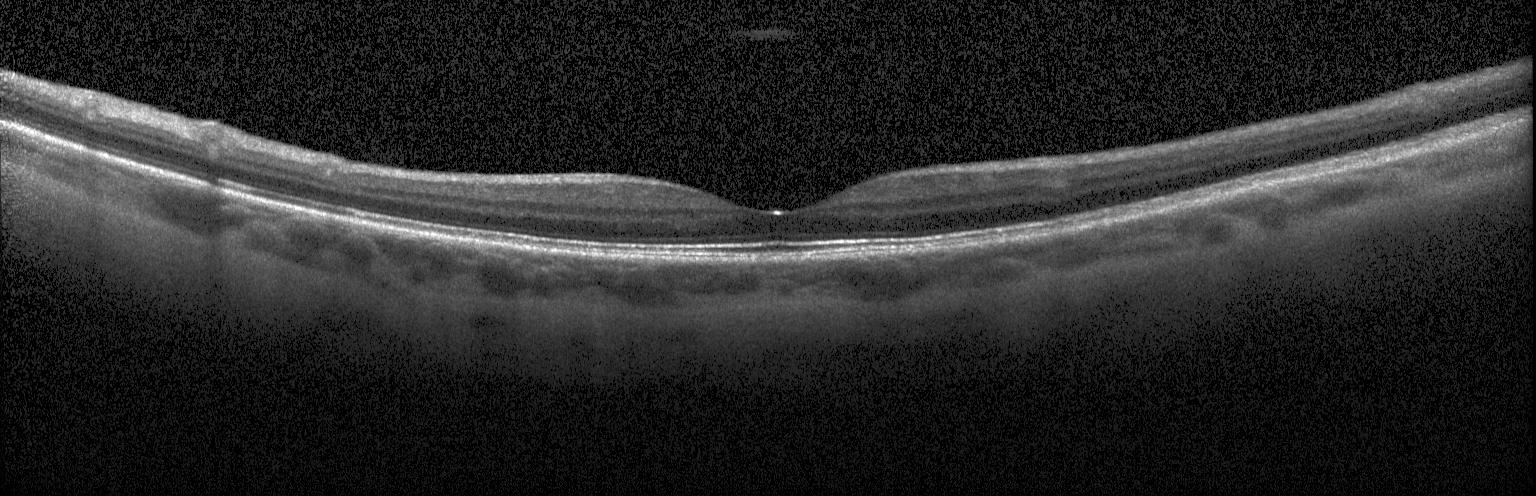

Finding: no CNV, no DME, and no drusen.